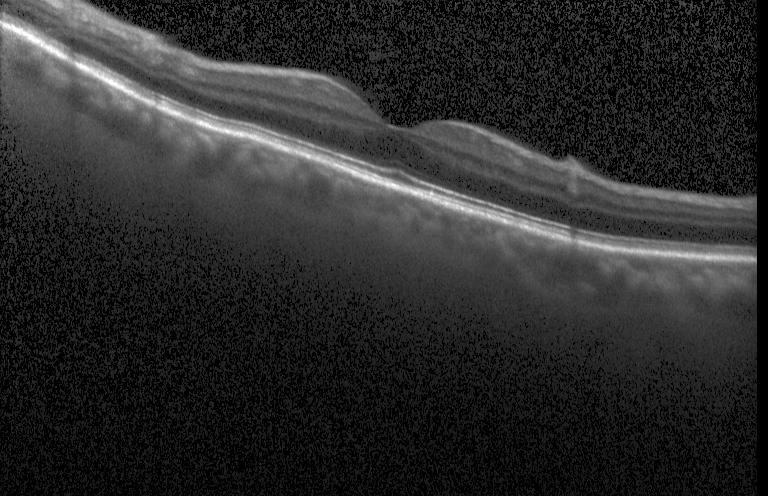 The scan shows no CNV, DME, or drusen.